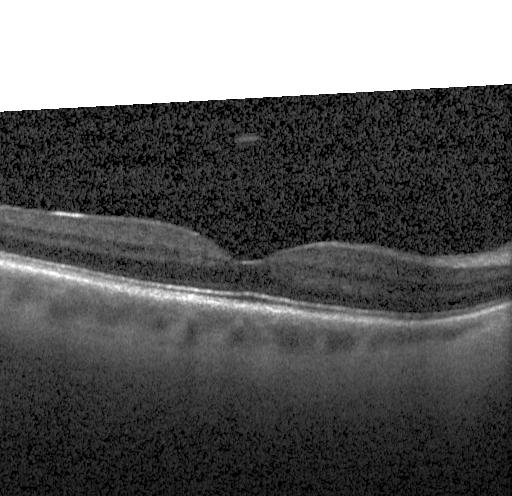
Impression: no choroidal neovascularization, diabetic macular edema, or drusen.